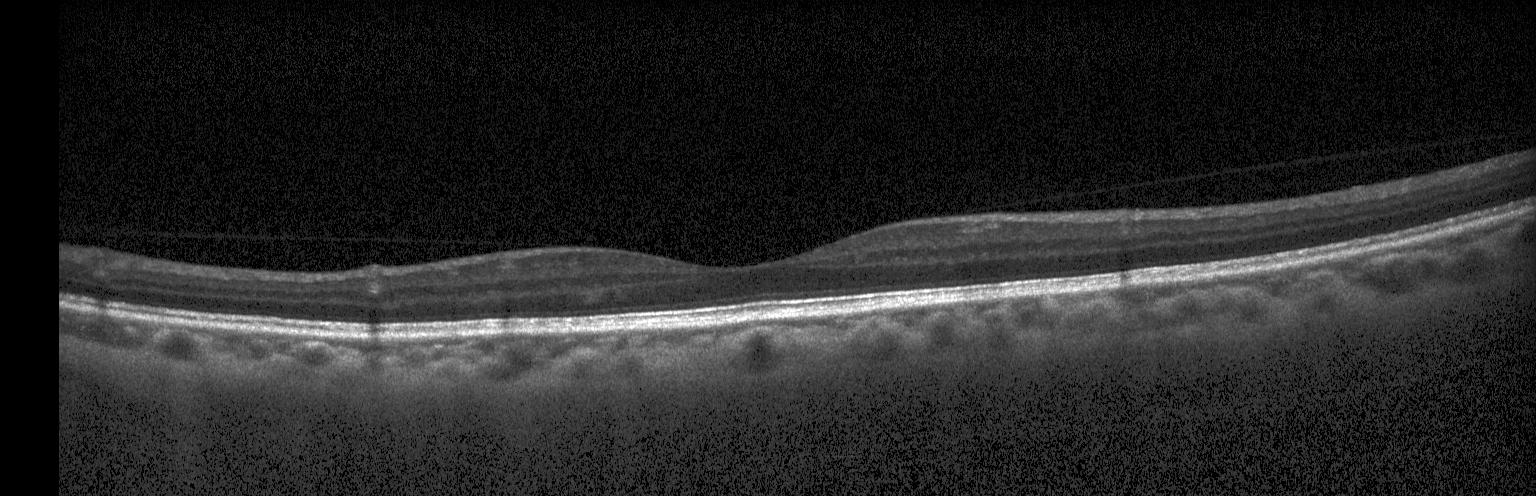 Optical coherence tomography scan, SD-OCT, macular scan
No CNV, no DME, and no drusen.